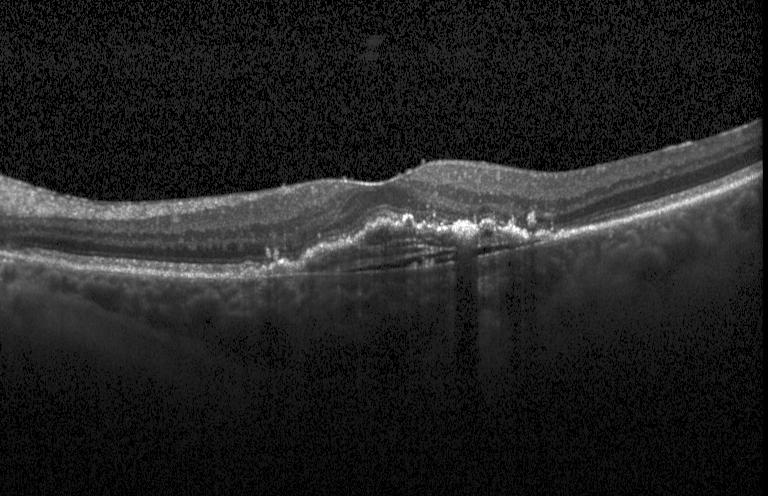 OCT B-scan
Choroidal neovascularization (CNV).